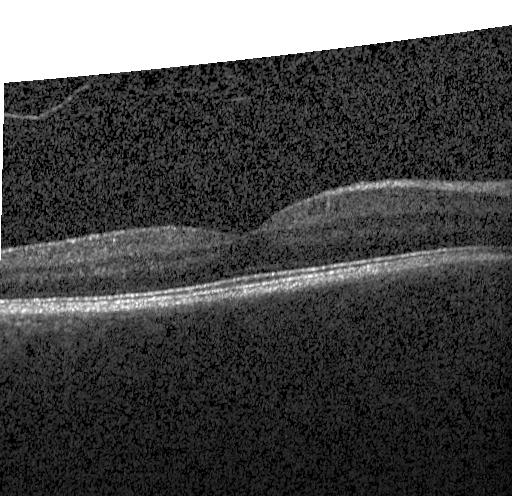
Through the macula. SD-OCT. Retinal OCT cross-section. Heidelberg Spectralis — OCT finding: no CNV, DME, or drusen.